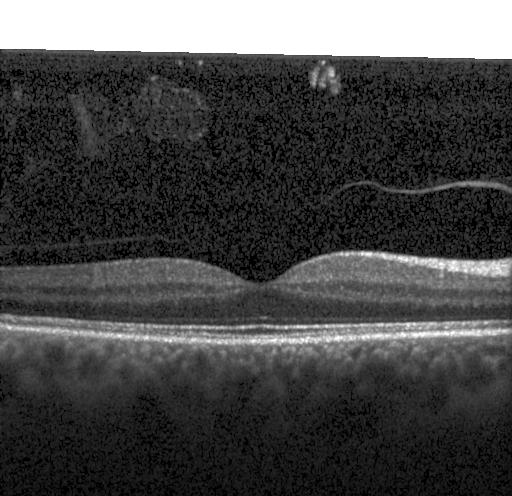 Fovea-centered; optical coherence tomography scan
Macular OCT: neither choroidal neovascularization, diabetic macular edema, nor drusen.